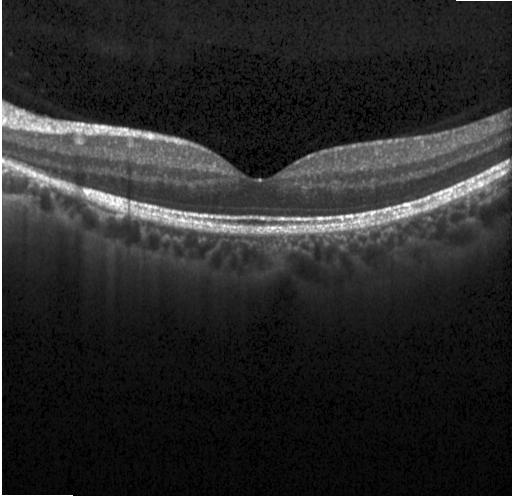 Finding: no choroidal neovascularization, no diabetic macular edema, and no drusen.